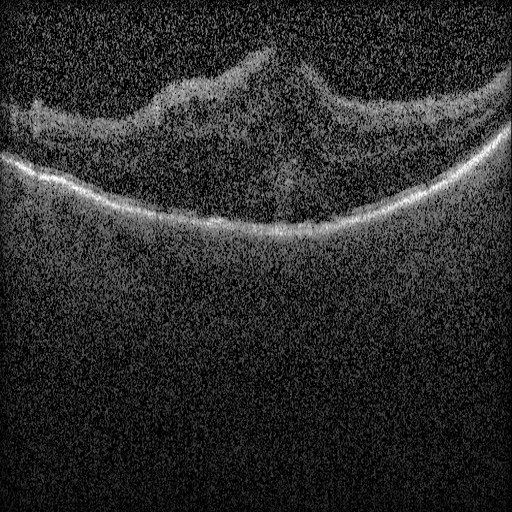
Spectral-domain OCT; optical coherence tomography scan.
OCT finding: diabetic macular edema (DME).